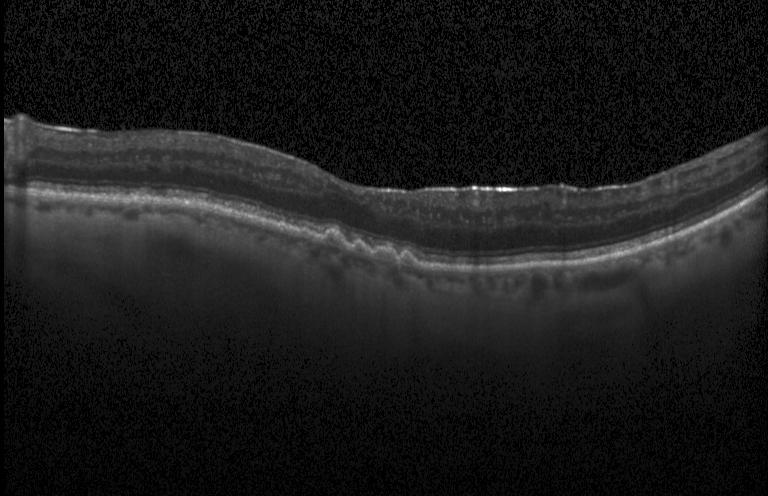 Impression: sub-RPE drusenoid deposits.